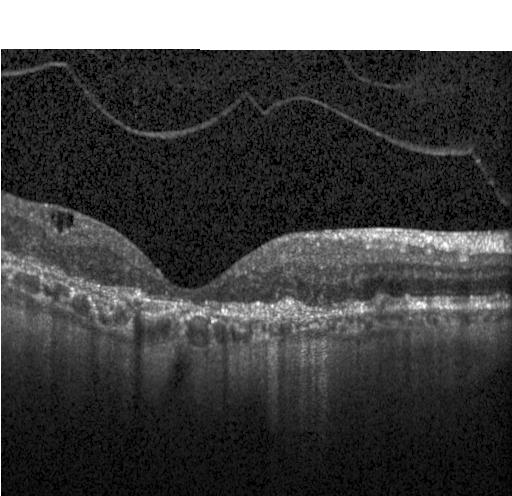
Macular scan. Heidelberg Spectralis. Optical coherence tomography B-scan. Dx: a choroidal neovascular membrane.